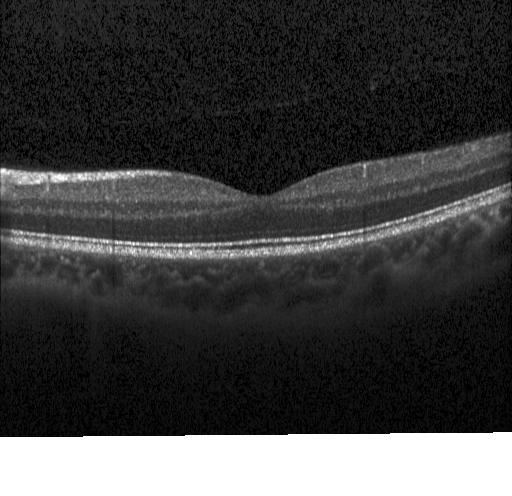 Impression: neither choroidal neovascularization, diabetic macular edema, nor drusen.